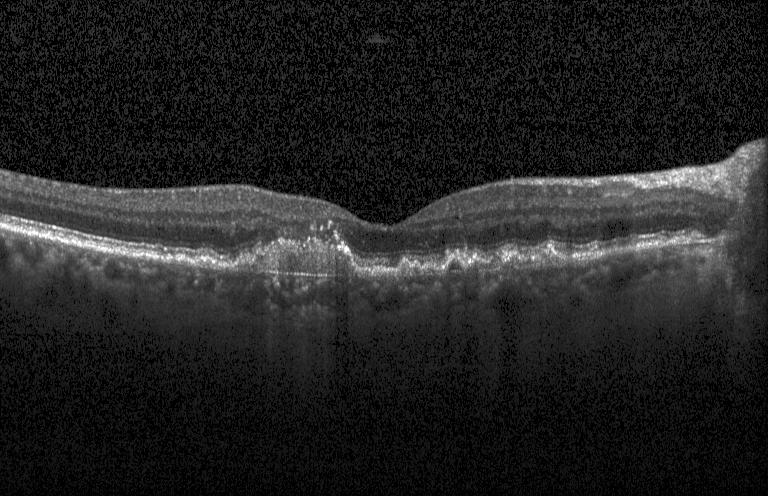

OCT B-scan, through the macula, Heidelberg Spectralis — Dx: choroidal neovascularization (CNV).